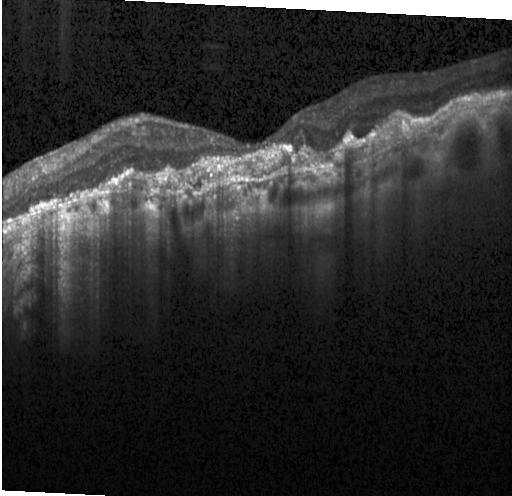 Spectral-domain OCT. Optical coherence tomography scan. Through the macula.
Assessment: choroidal neovascularization.